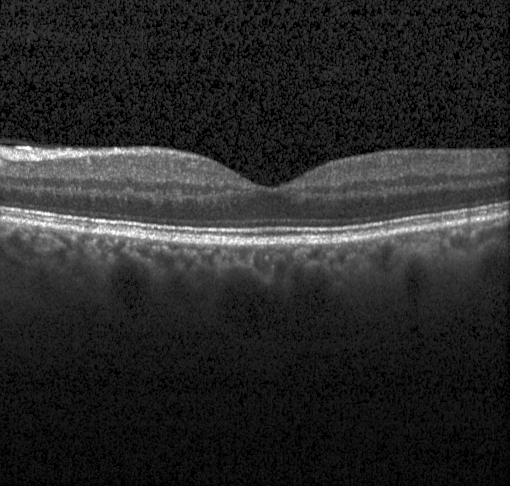 Diagnosis: no choroidal neovascularization, no diabetic macular edema, and no drusen.